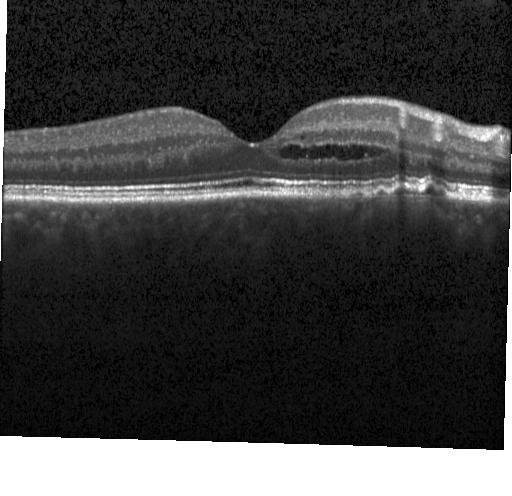 Through the macula, SD-OCT, optical coherence tomography scan, acquired on a Heidelberg Spectralis
Impression: CNV.